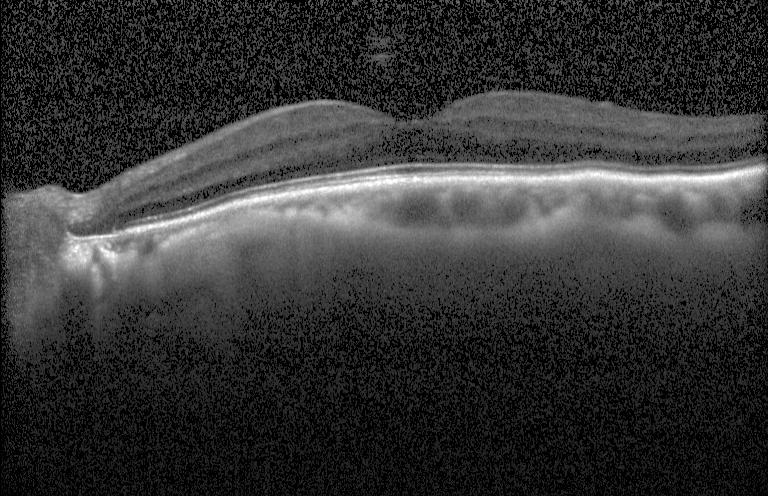
OCT B-scan showing no CNV, DME, or drusen.